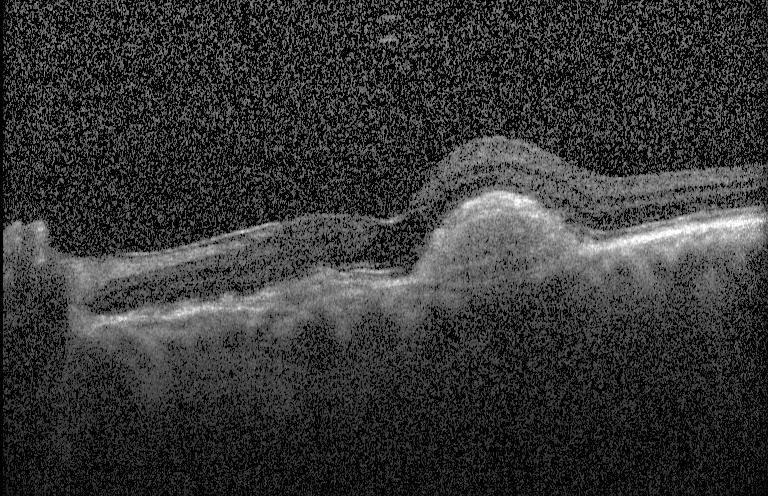 The scan shows a choroidal neovascular membrane.